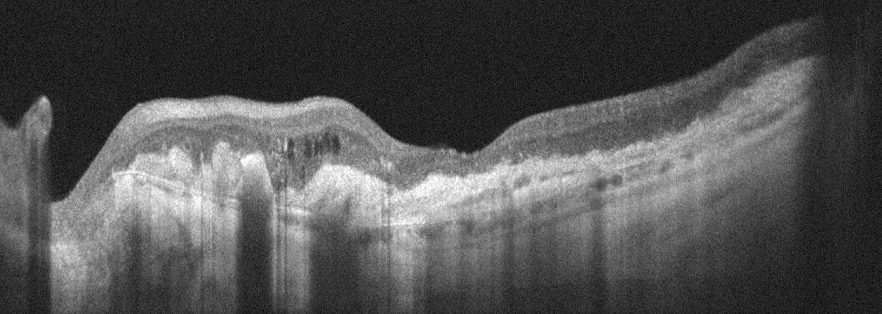

Acquired on an Optovue Avanti RTVue XR, optical coherence tomography scan, through the macula, left eye. Diagnosis: AMD.